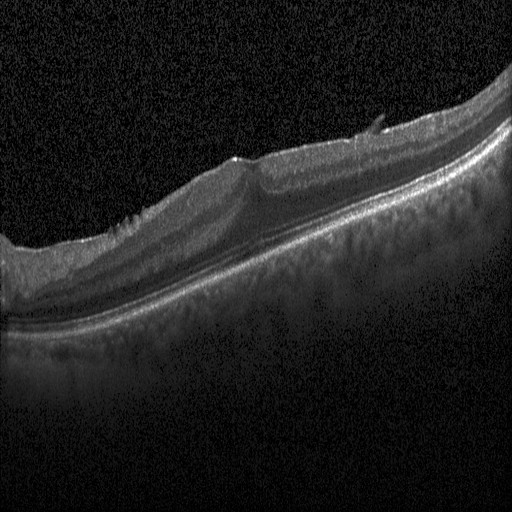

Optical coherence tomography scan. Diagnosis: diabetic macular edema.